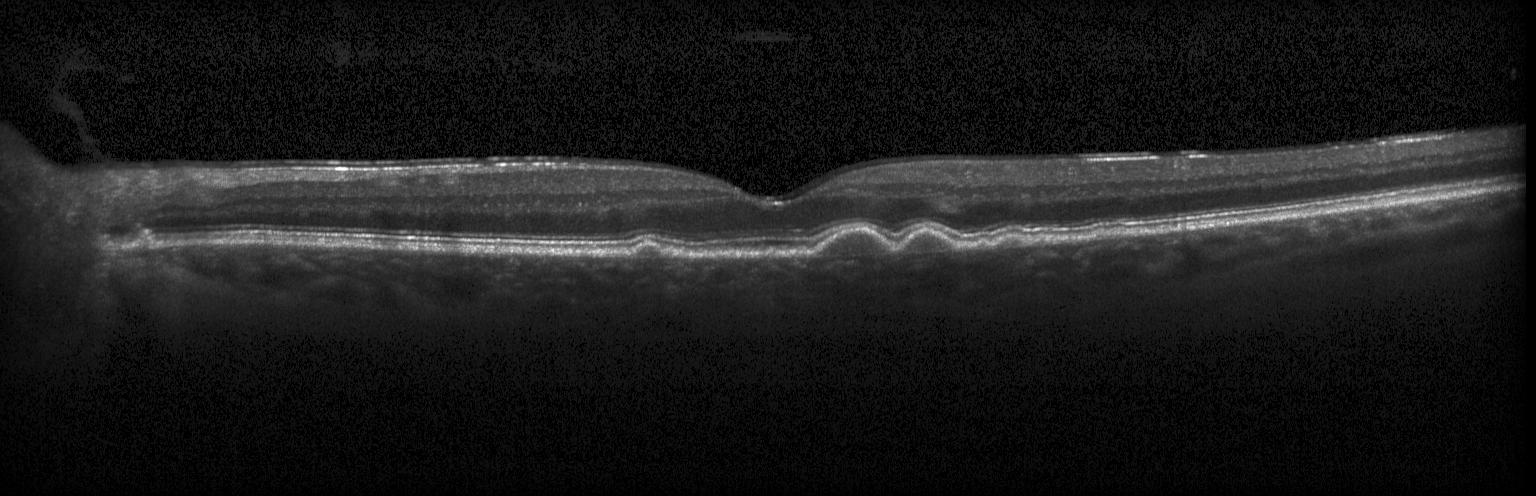
Optical coherence tomography B-scan, through the macula, spectral-domain optical coherence tomography, Heidelberg Spectralis OCT system
OCT finding: multiple drusen.